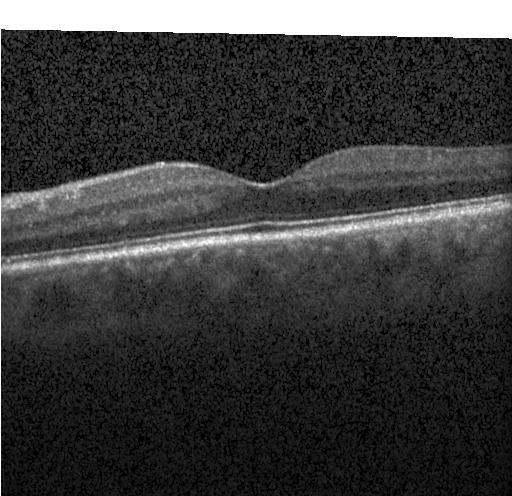 Spectral-domain OCT · fovea-centered · optical coherence tomography scan · Heidelberg Spectralis OCT system.
Finding: no choroidal neovascularization, no diabetic macular edema, and no drusen.